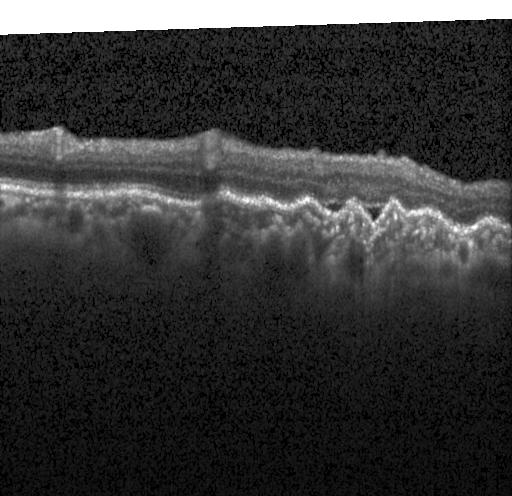

Impression: choroidal neovascularization.